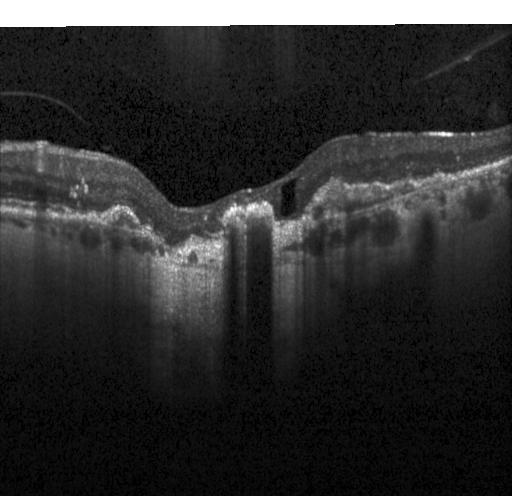 This B-scan demonstrates CNV.